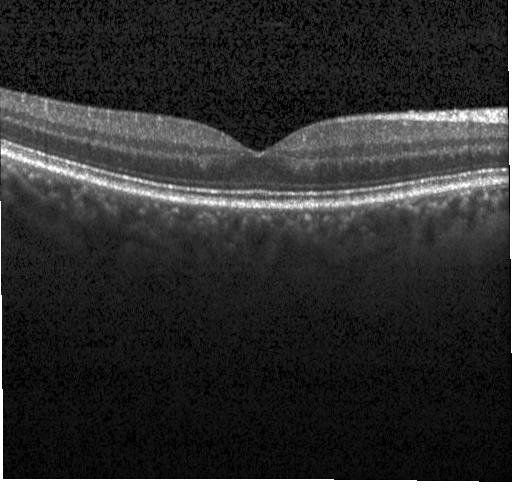 The scan shows no evidence of CNV, DME, or drusen.